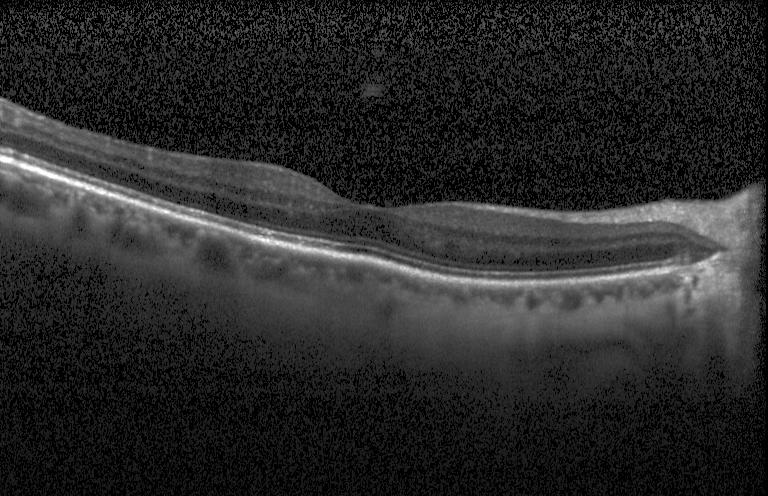 OCT B-scan. Assessment: no choroidal neovascularization, no diabetic macular edema, and no drusen.